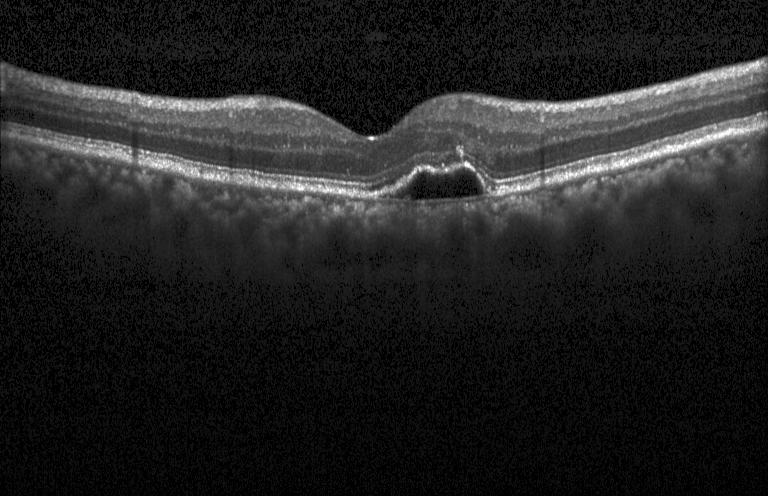

Macular scan; OCT B-scan
Finding: choroidal neovascularization.